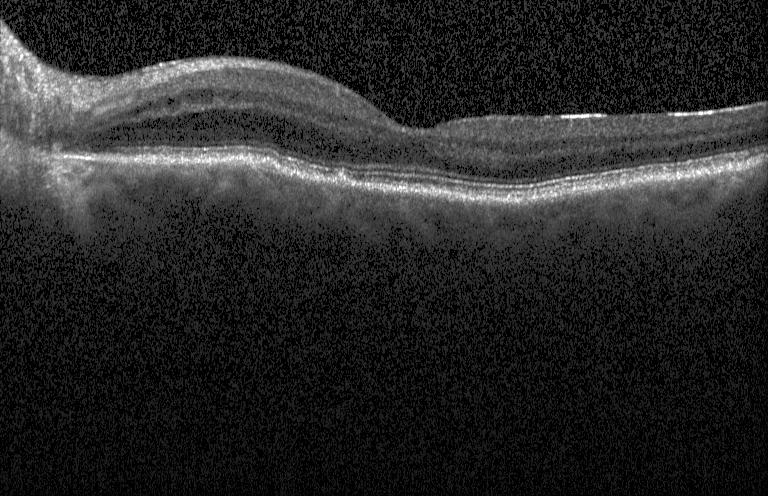 Finding: drusen.